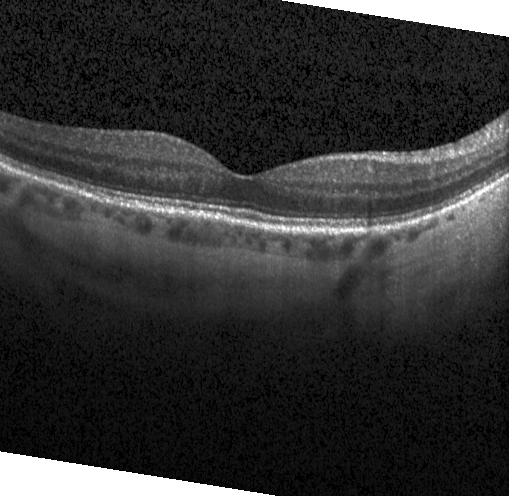

Retinal OCT B-scan. Spectral-domain OCT. Heidelberg Spectralis. Horizontal scan through the fovea — Diagnosis: no CNV, DME, or drusen.